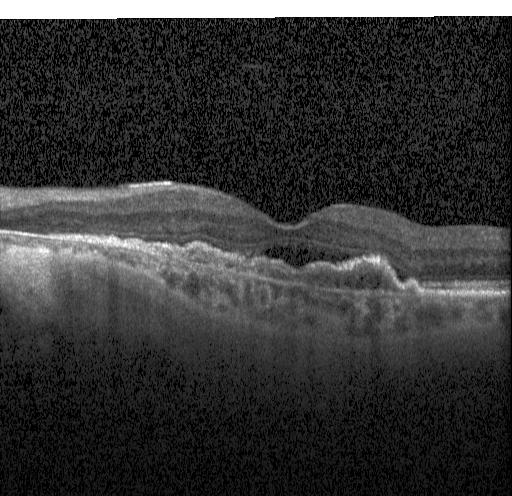 OCT line scan. Horizontal scan through the fovea. Choroidal neovascularization (CNV).